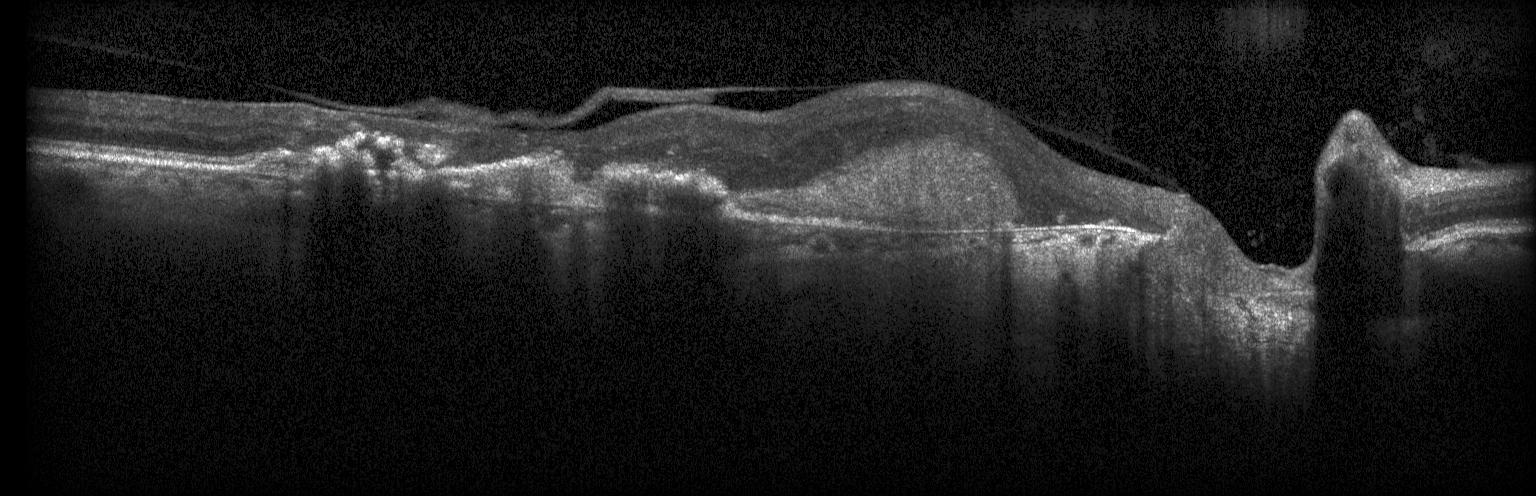
Spectral-domain optical coherence tomography · macular scan · optical coherence tomography scan — Impression: a choroidal neovascular membrane.